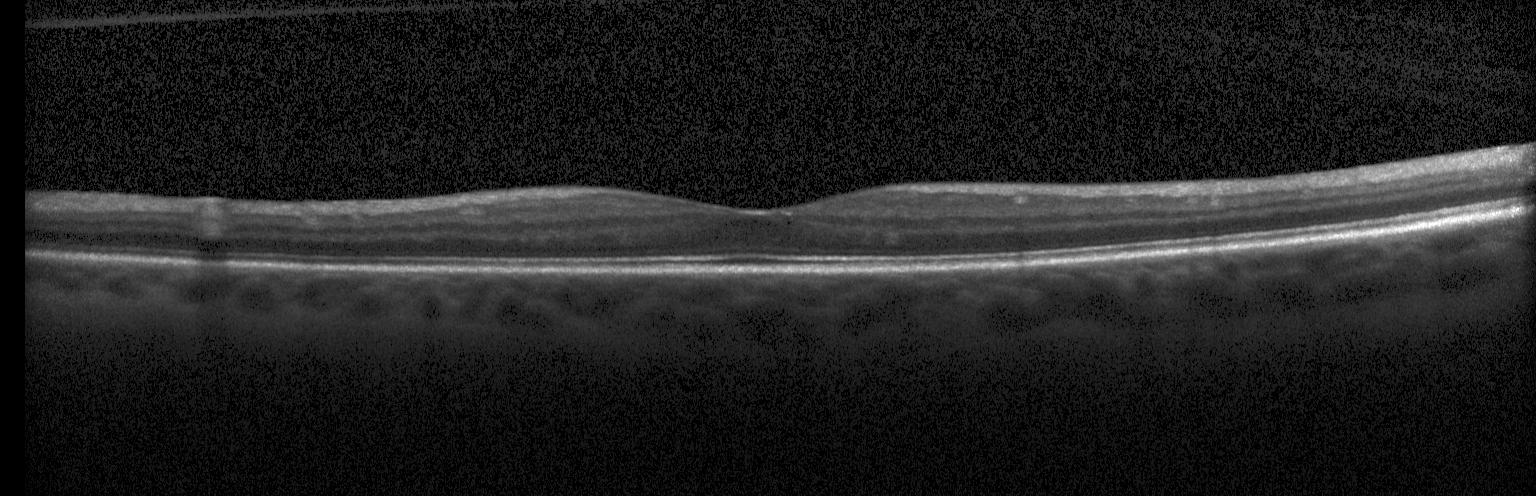

Retinal OCT B-scan · spectral-domain OCT
This B-scan demonstrates no evidence of choroidal neovascularization, diabetic macular edema, or drusen.